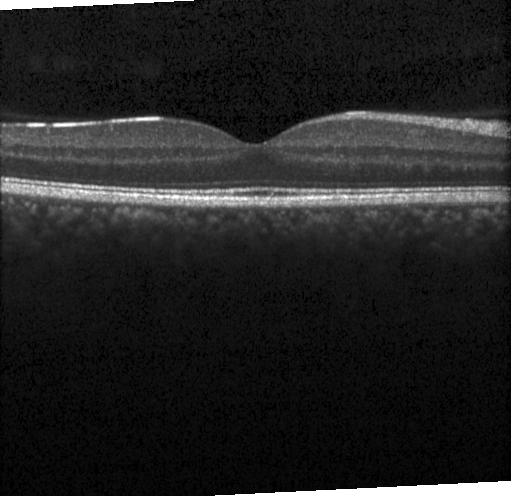 Diagnosis: no choroidal neovascularization, diabetic macular edema, or drusen.